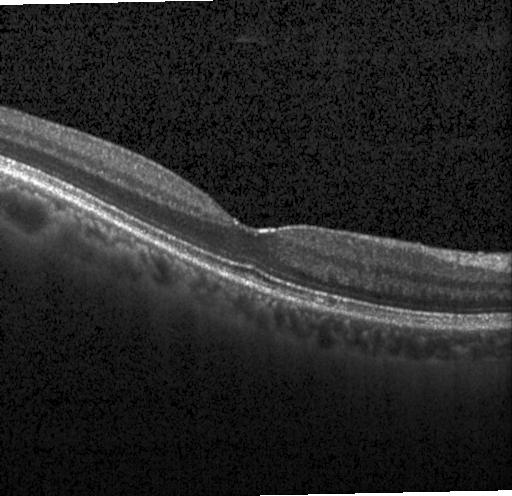 Diagnosis: no choroidal neovascularization, no diabetic macular edema, and no drusen.